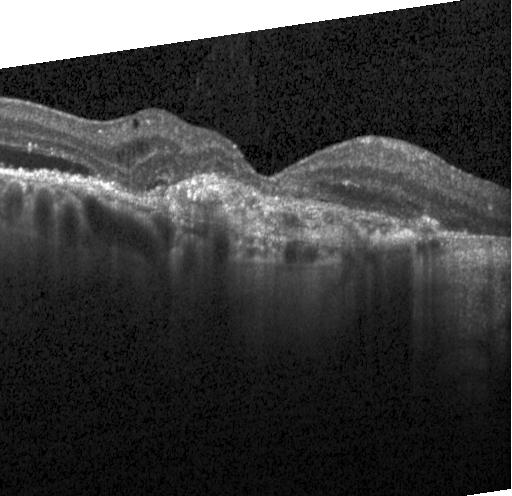 OCT line scan; horizontal scan through the fovea; spectral-domain optical coherence tomography
Finding: choroidal neovascularization (CNV).